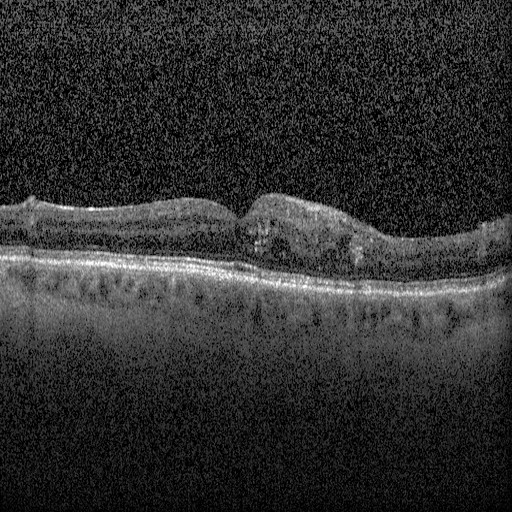
Assessment: diabetic macular edema (DME).